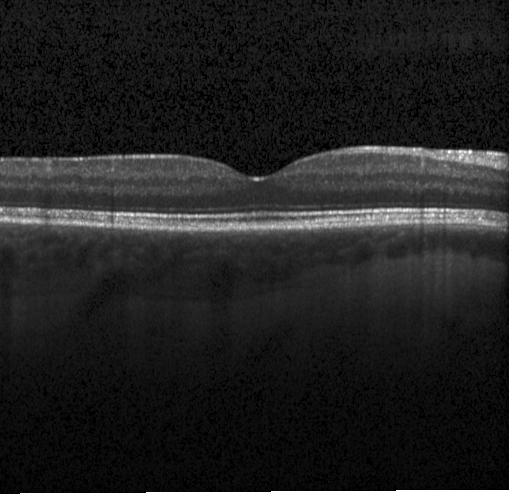

OCT B-scan — Macular OCT: no choroidal neovascularization, diabetic macular edema, or drusen.